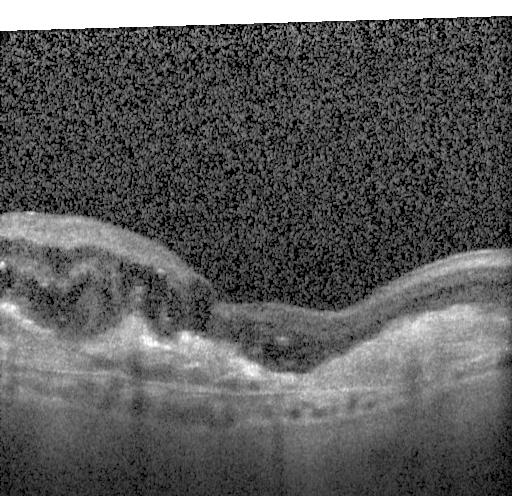 Centered on the fovea, Heidelberg Spectralis, spectral-domain OCT, OCT line scan.
The scan shows CNV.